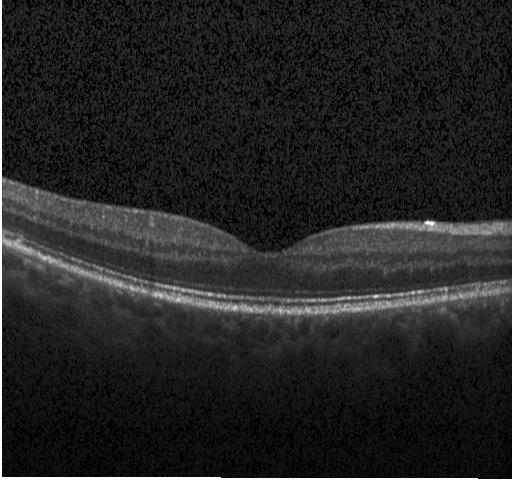 Finding: no choroidal neovascularization, no diabetic macular edema, and no drusen.